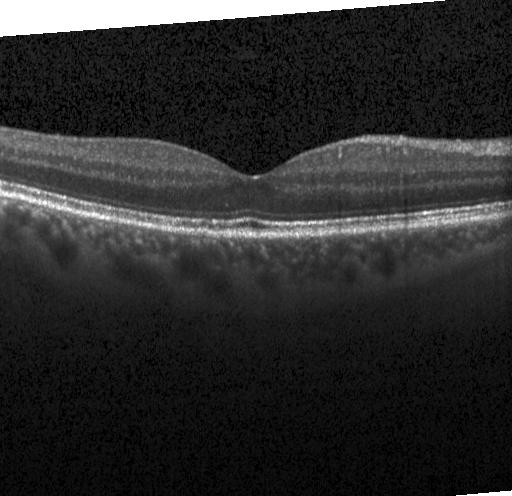
Spectral-domain OCT, instrument: Heidelberg Spectralis, through the macula, retinal OCT cross-section. Assessment: no evidence of choroidal neovascularization, diabetic macular edema, or drusen.